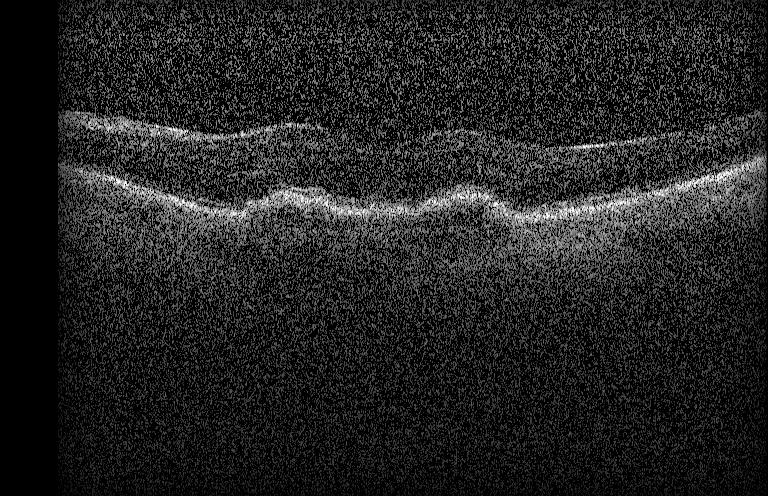
SD-OCT · Heidelberg Spectralis OCT system · centered on the fovea · retinal OCT B-scan
OCT finding: choroidal neovascularization.